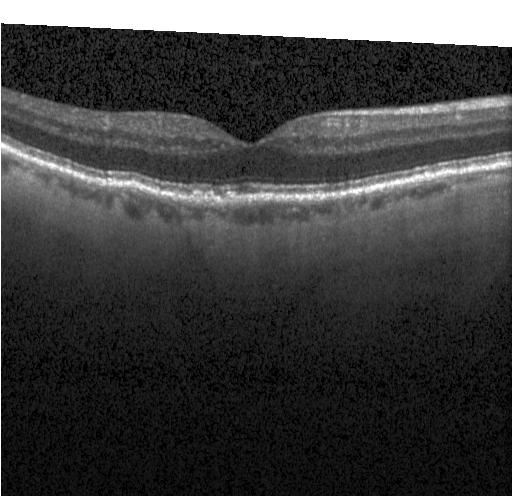 Optical coherence tomography scan. Finding: sub-RPE drusenoid deposits.